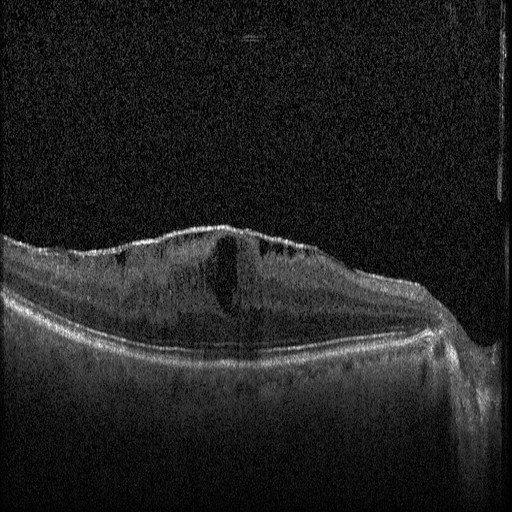

Diagnosis: DME.